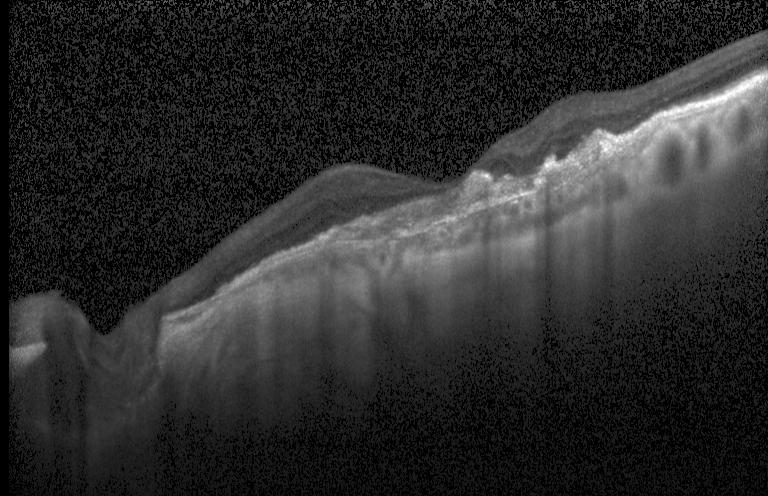

Spectral-domain OCT B-scan: a choroidal neovascular membrane.